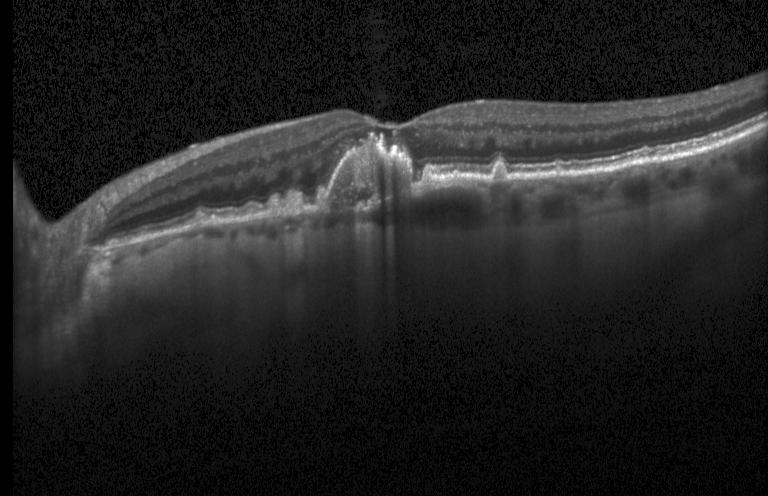

OCT scan showing choroidal neovascularization.